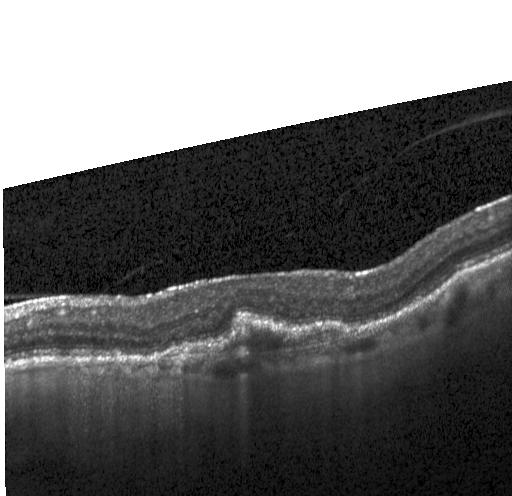

Macular OCT: a choroidal neovascular membrane.